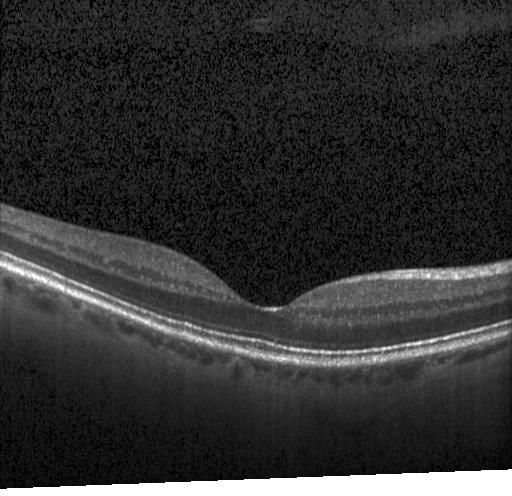
OCT B-scan; fovea-centered
Finding: no CNV, no DME, and no drusen.